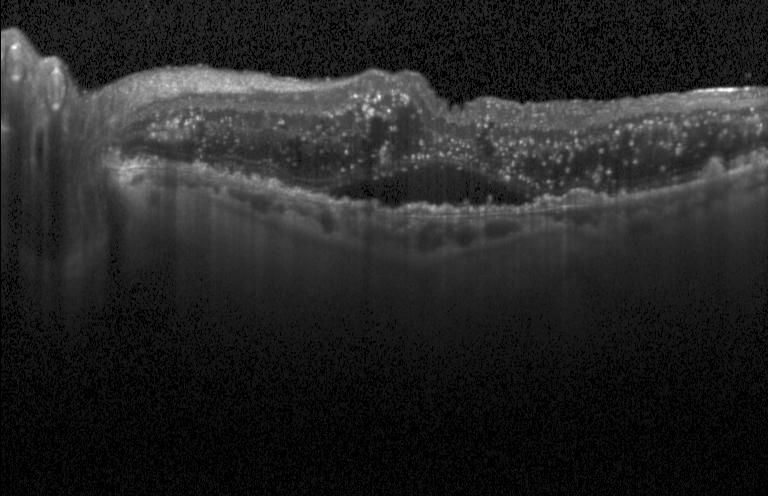

Instrument: Heidelberg Spectralis, optical coherence tomography B-scan
Finding: a choroidal neovascular membrane.